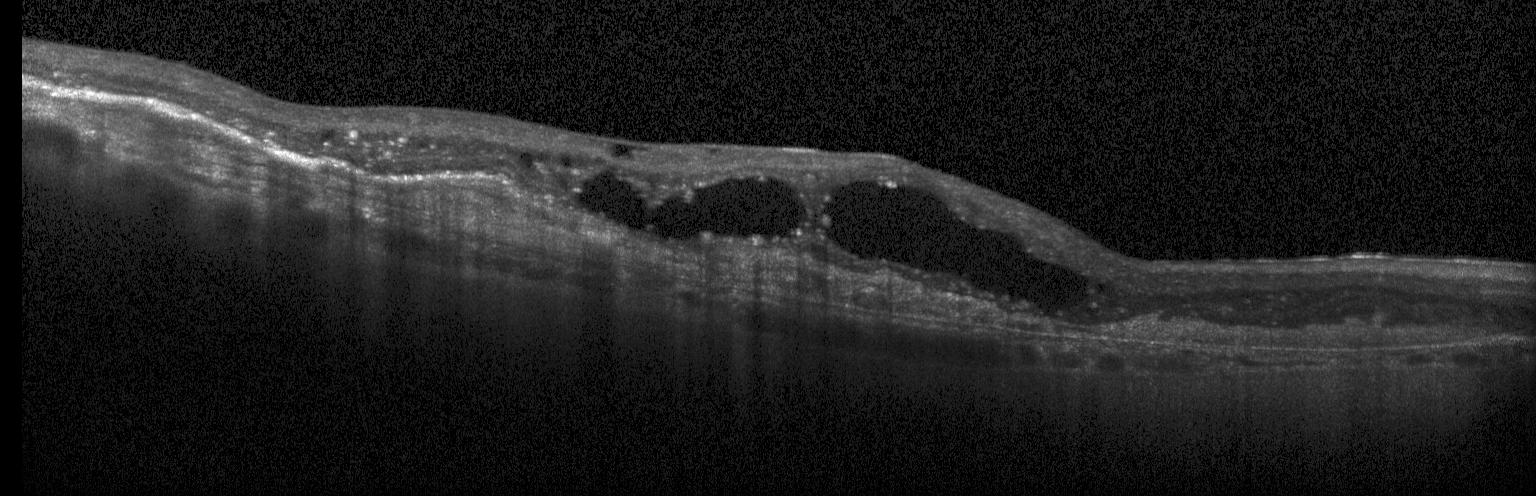 Horizontal scan through the fovea; retinal OCT cross-section.
OCT finding: a choroidal neovascular membrane.